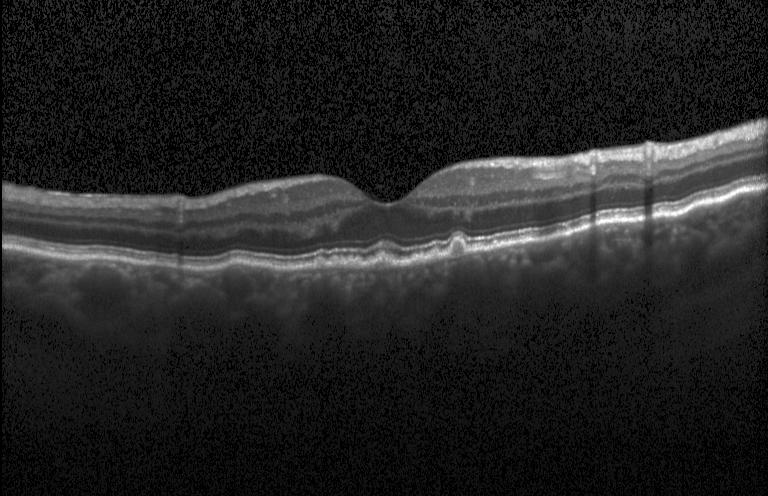

OCT line scan, centered on the fovea, Heidelberg Spectralis OCT system. Finding: multiple drusen.